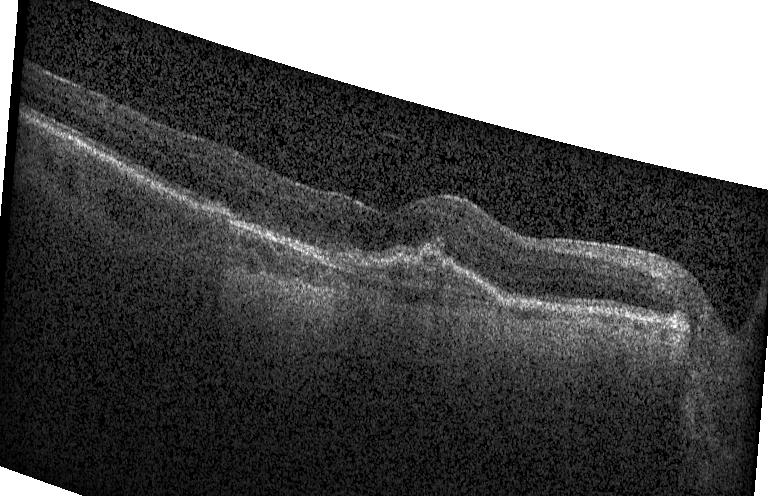

Macular scan; OCT line scan.
Impression: choroidal neovascularization (CNV).